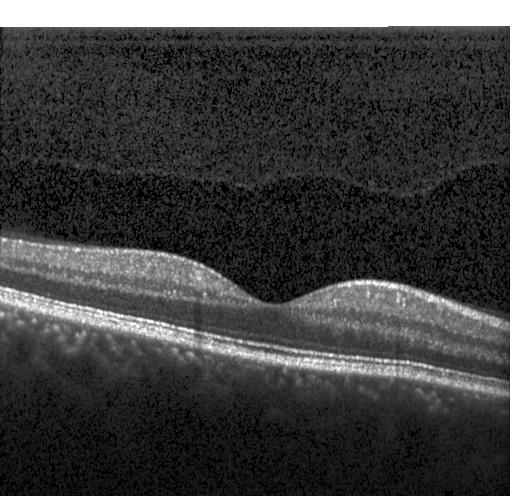 Diagnosis: no CNV, DME, or drusen.